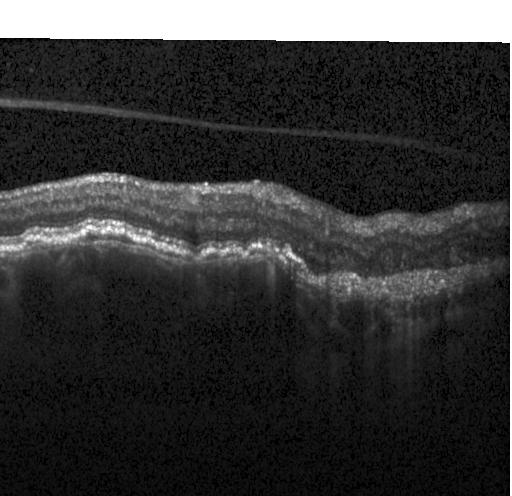

Through the macula. Acquired on a Heidelberg Spectralis. Retinal OCT cross-section. The scan shows a choroidal neovascular membrane.